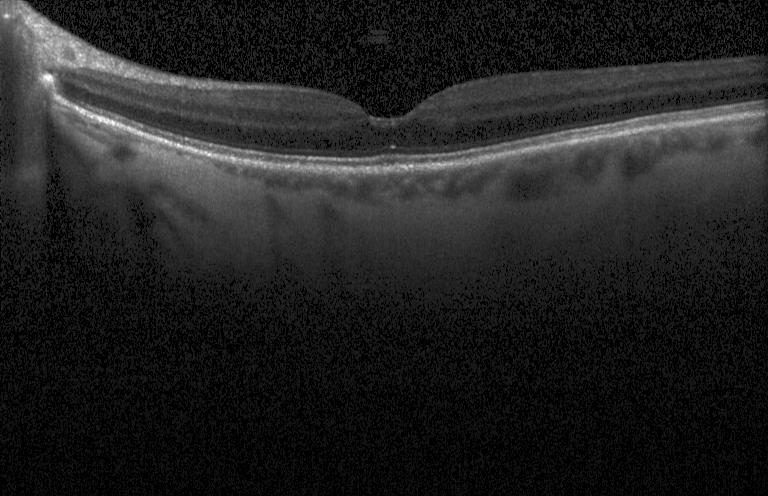
Impression: no evidence of CNV, DME, or drusen.